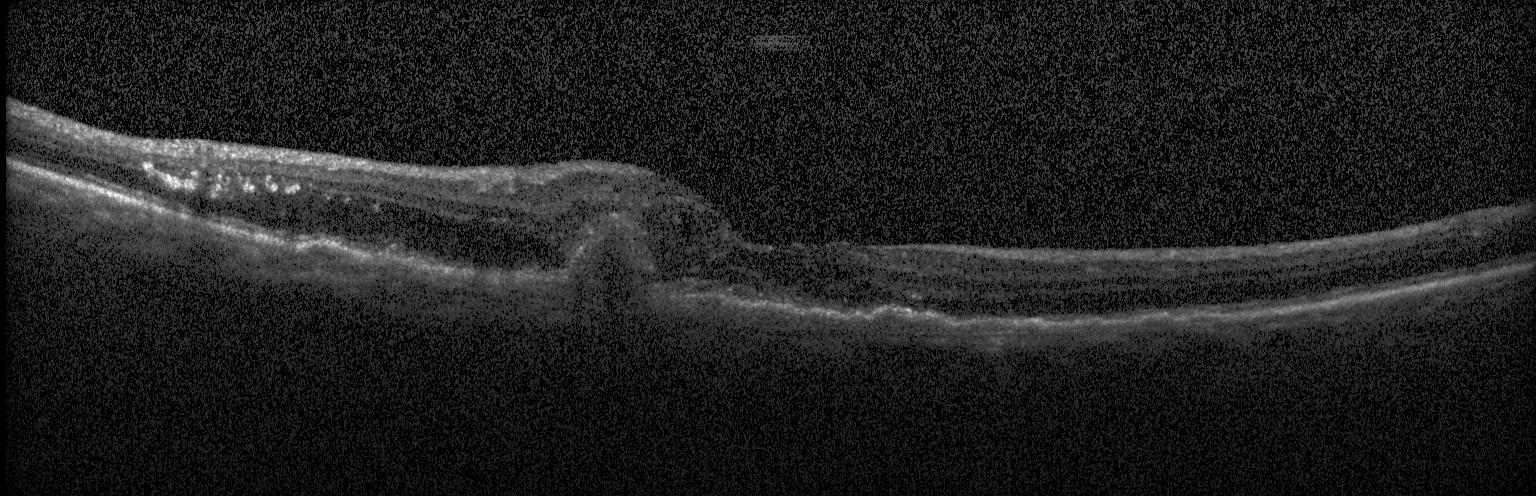

Spectral-domain OCT B-scan: a choroidal neovascular membrane.